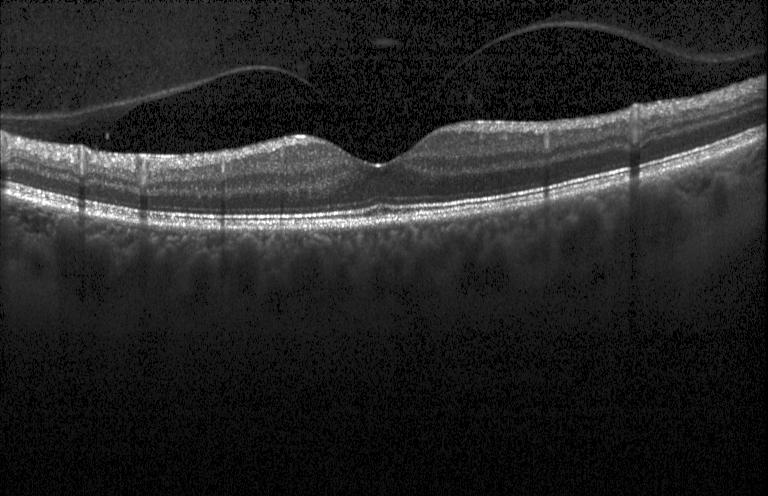

OCT line scan — Diagnosis: no choroidal neovascularization, no diabetic macular edema, and no drusen.